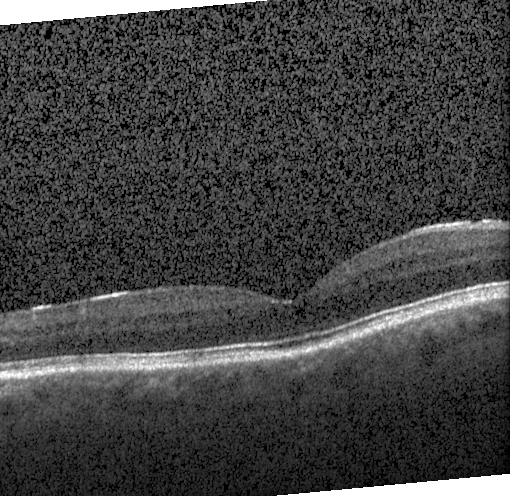

OCT B-scan.
This B-scan demonstrates no evidence of CNV, DME, or drusen.